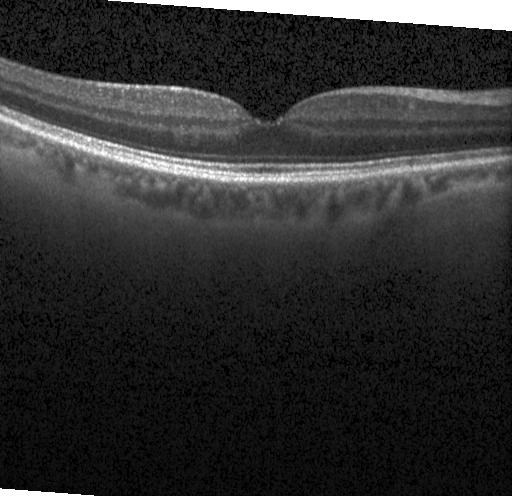 Spectral-domain OCT · optical coherence tomography scan · macular scan · instrument: Heidelberg Spectralis.
Assessment: no evidence of CNV, DME, or drusen.